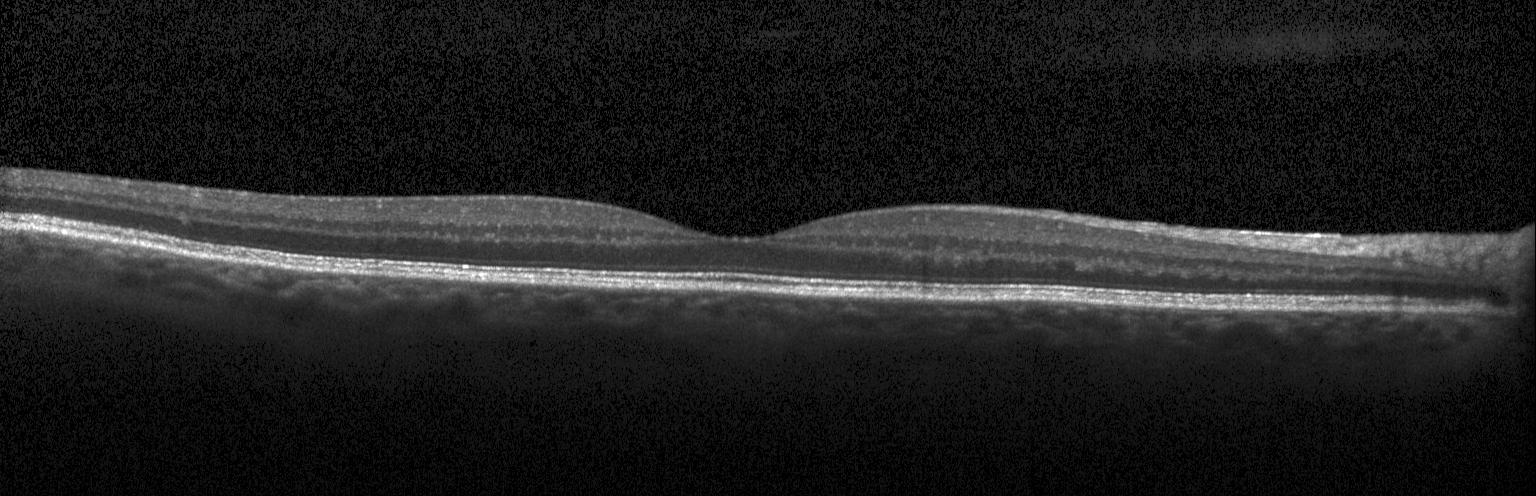
Finding: neither CNV, DME, nor drusen.